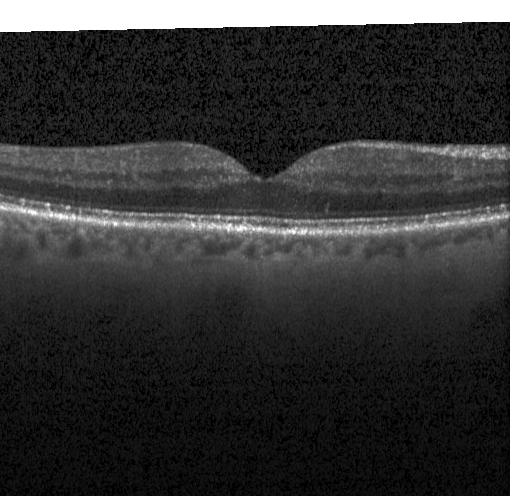 Retinal OCT cross-section. Macular OCT: no evidence of choroidal neovascularization, diabetic macular edema, or drusen.